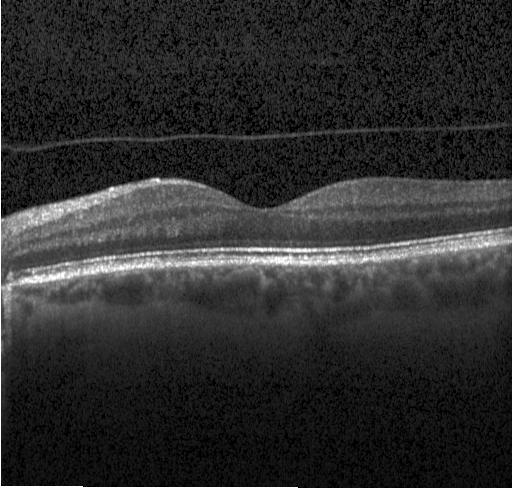 Retinal OCT B-scan; centered on the fovea. Assessment: no choroidal neovascularization, diabetic macular edema, or drusen.